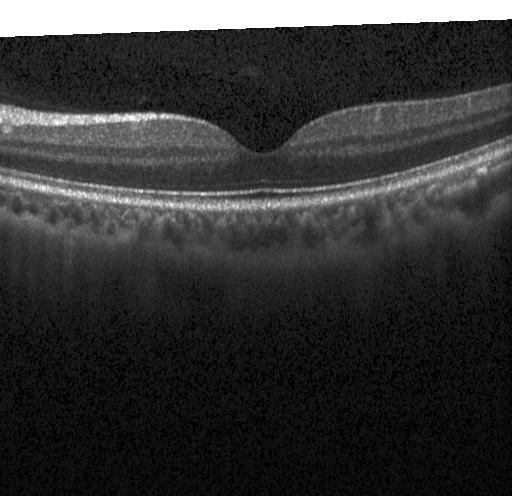 Spectral-domain optical coherence tomography · OCT line scan · through the macula.
Diagnosis: neither choroidal neovascularization, diabetic macular edema, nor drusen.